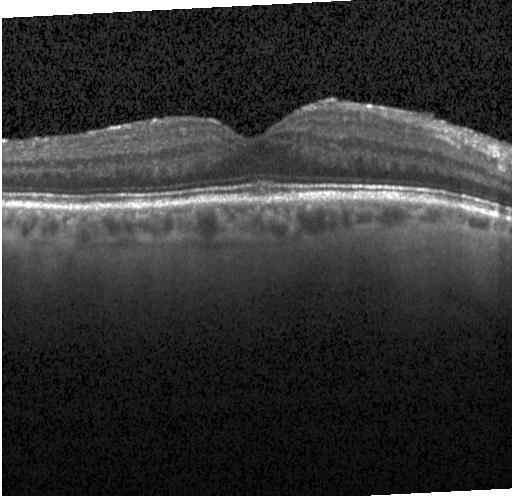 Diagnosis: no evidence of choroidal neovascularization, diabetic macular edema, or drusen.